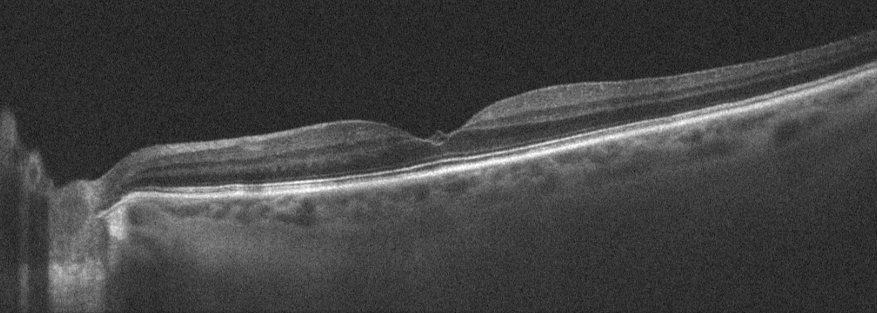

Impression: absence of AMD, DME, ERM, RAO, RVO, and vitreomacular interface disease.